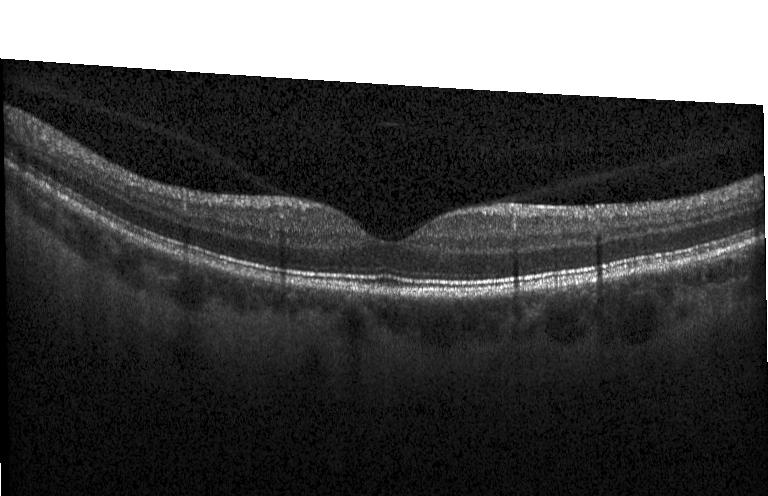 Retinal OCT B-scan. Fovea-centered. Heidelberg Spectralis OCT system — Assessment: no evidence of CNV, DME, or drusen.